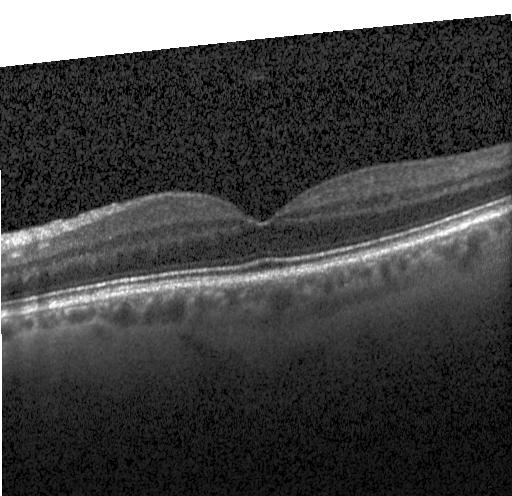
Optical coherence tomography B-scan — This B-scan demonstrates no CNV, no DME, and no drusen.